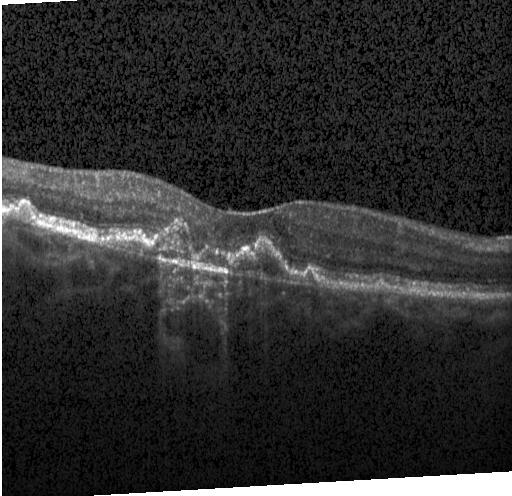

Impression: choroidal neovascularization.